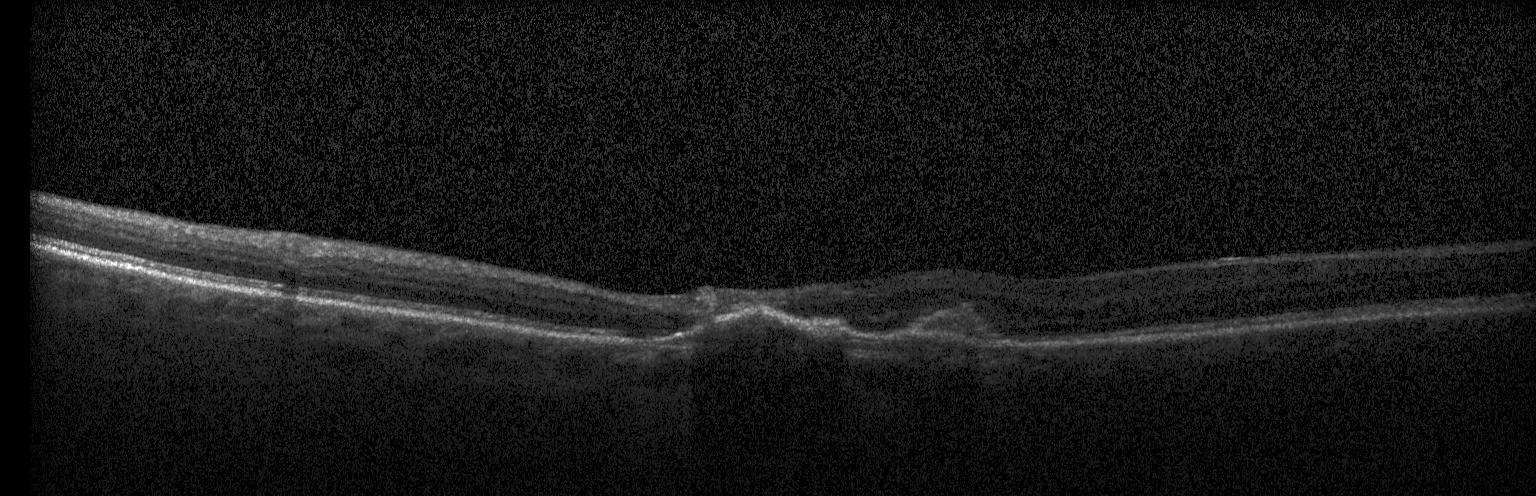
Fovea-centered, spectral-domain optical coherence tomography, retinal OCT B-scan. Finding: CNV.